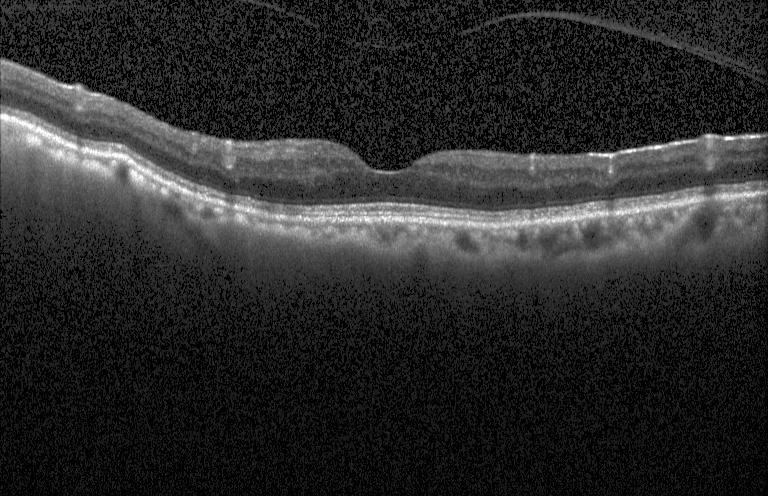
Retinal OCT B-scan — Macular OCT: neither choroidal neovascularization, diabetic macular edema, nor drusen.